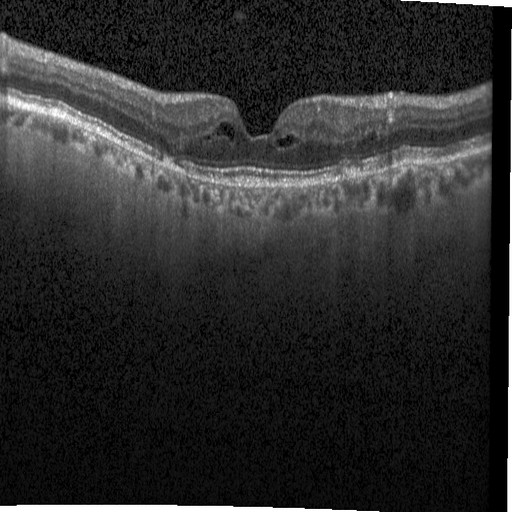 OCT B-scan
Impression: diabetic macular edema.